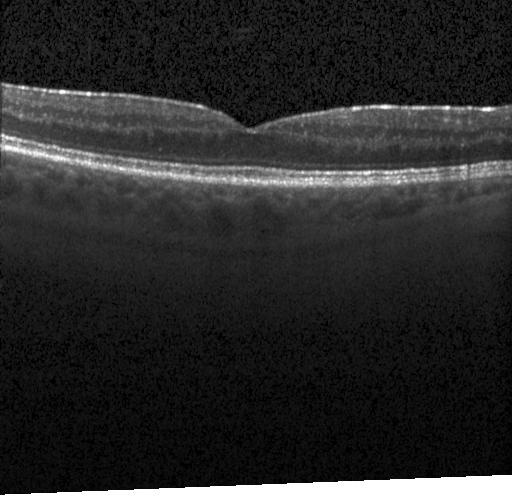 Spectral-domain OCT. Retinal OCT B-scan. Acquired on a Heidelberg Spectralis. Centered on the fovea
Dx: no evidence of choroidal neovascularization, diabetic macular edema, or drusen.